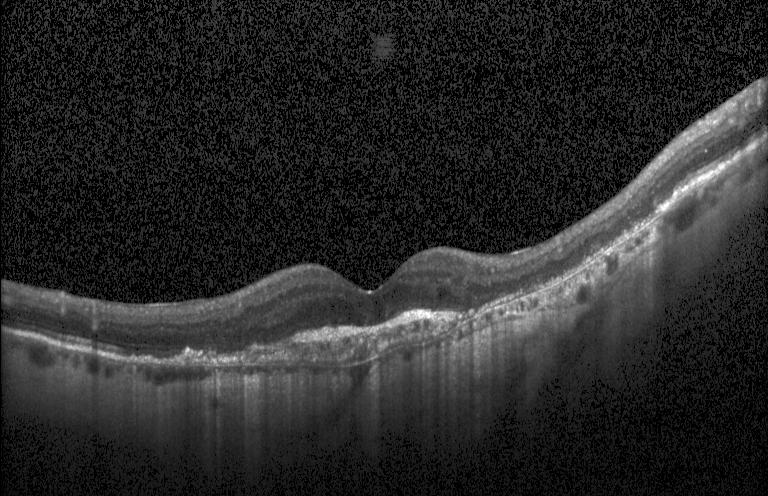

This B-scan demonstrates a choroidal neovascular membrane.